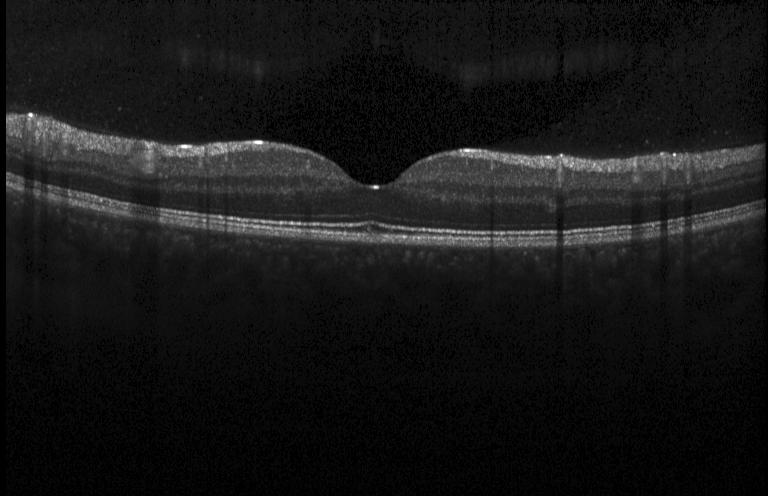
Macular OCT: no CNV, DME, or drusen.